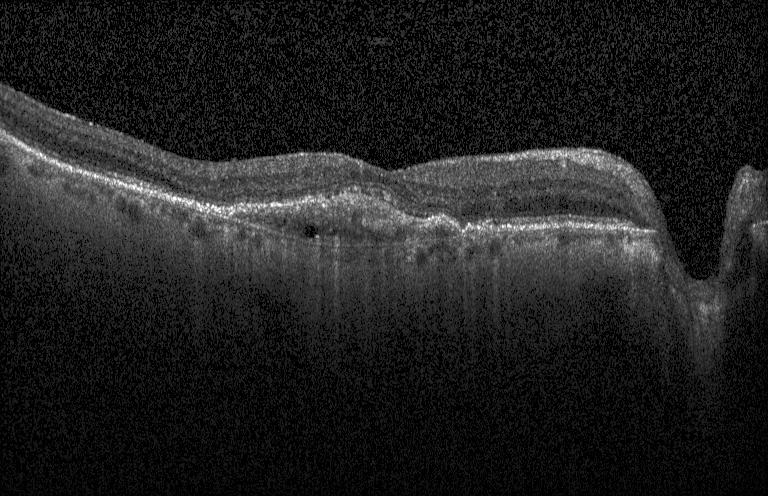
Optical coherence tomography B-scan
Assessment: CNV.